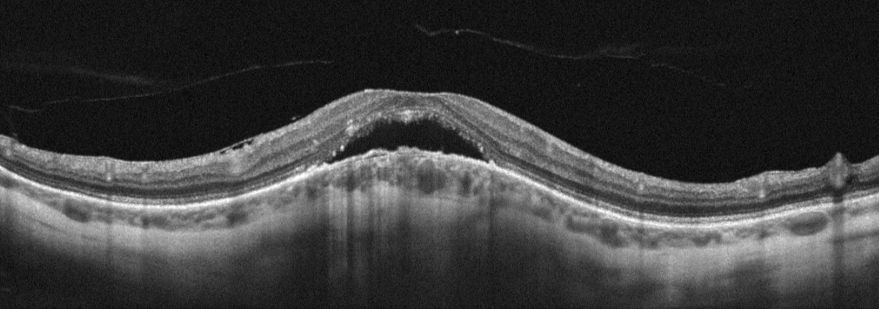

Acquired on an Optovue Avanti RTVue XR · through the macula · OCT B-scan — Dx: age-related macular degeneration (AMD).